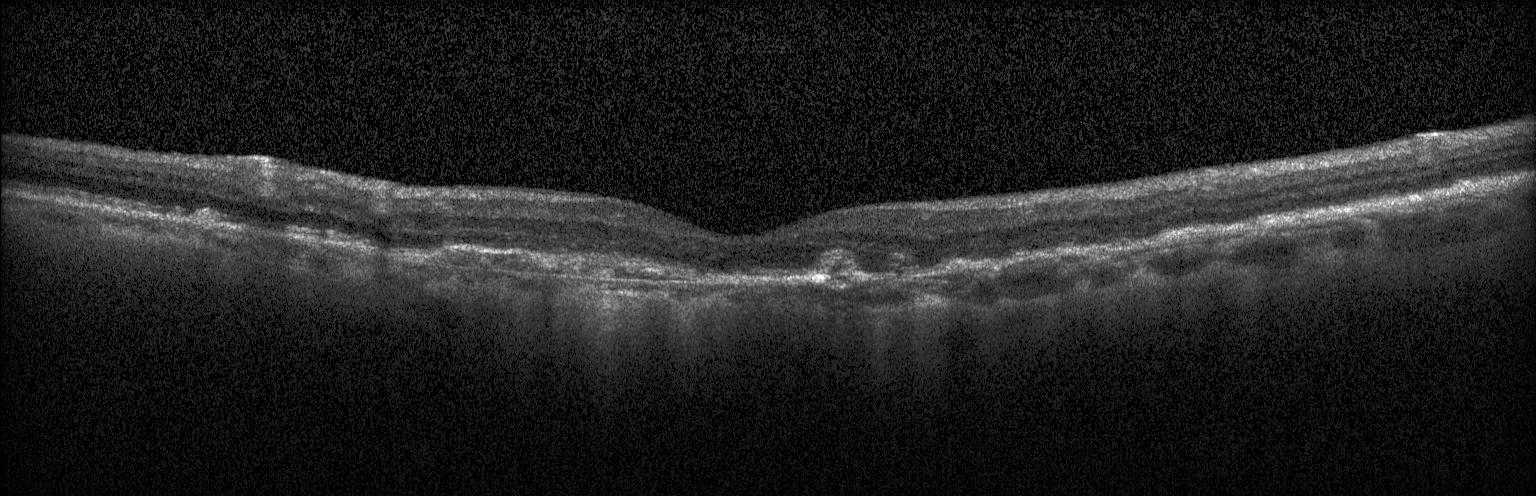
Diagnosis: CNV.